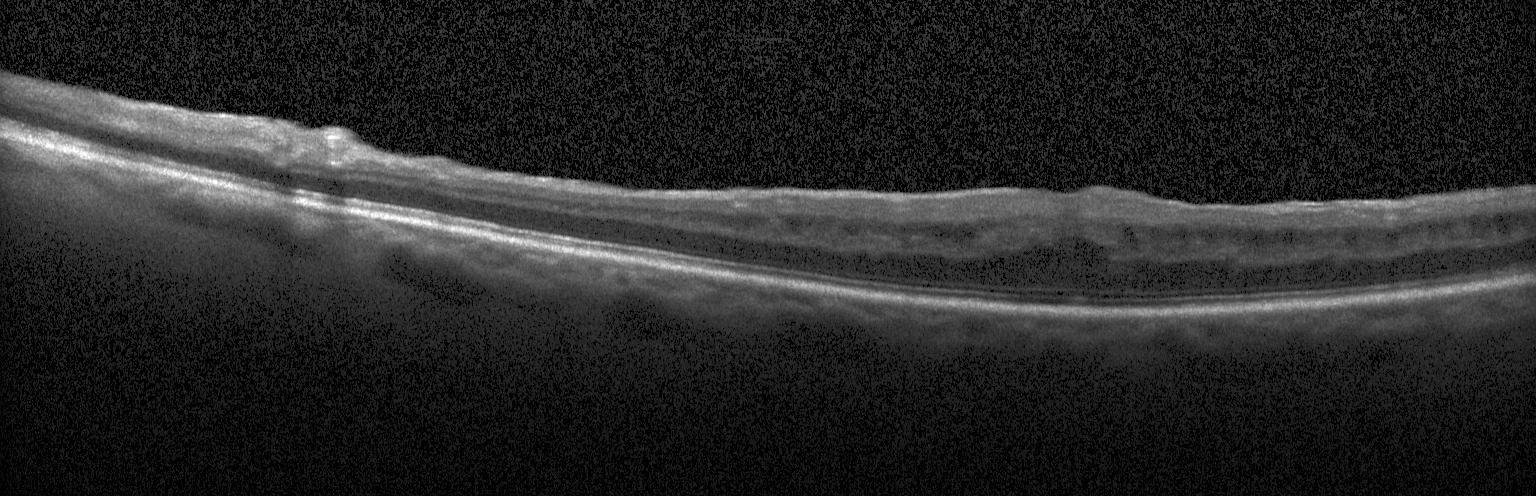

OCT finding: DME.